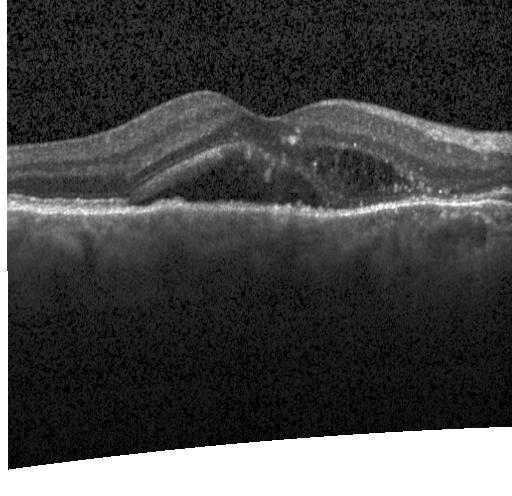 The scan shows choroidal neovascularization.